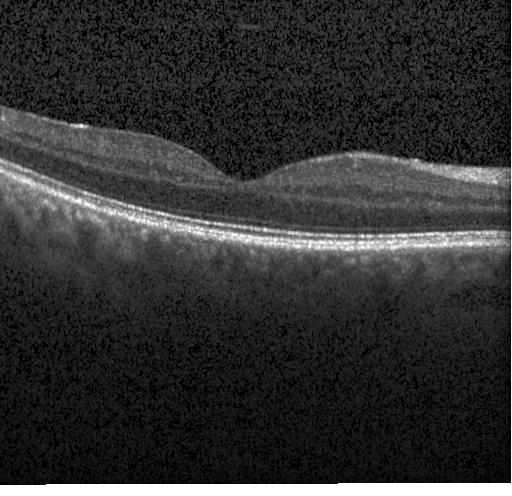 Optical coherence tomography scan.
Impression: neither choroidal neovascularization, diabetic macular edema, nor drusen.